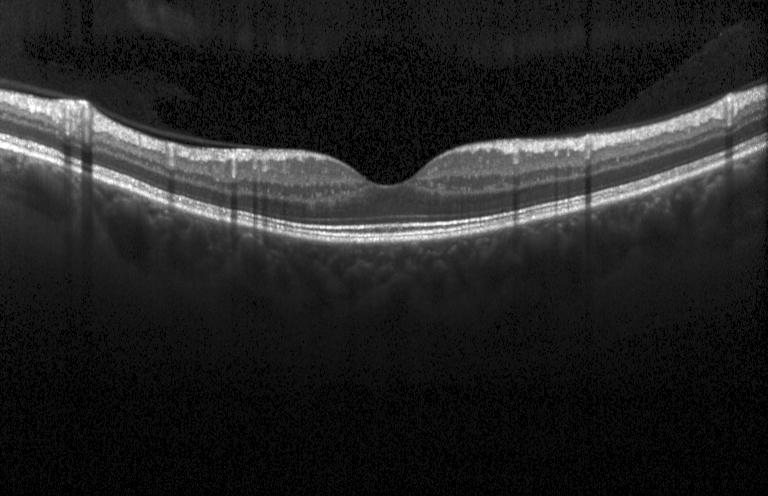

No choroidal neovascularization, diabetic macular edema, or drusen.